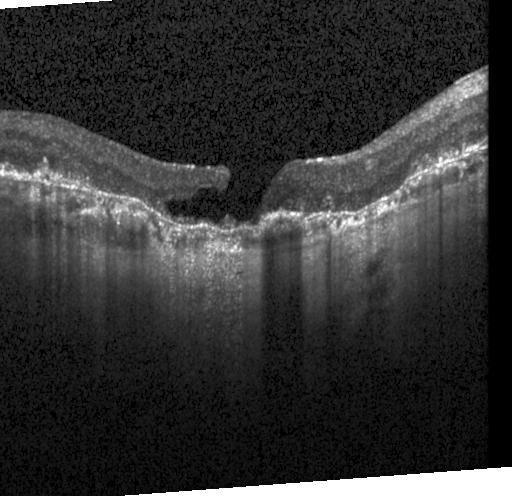 Macular OCT demonstrating choroidal neovascularization.